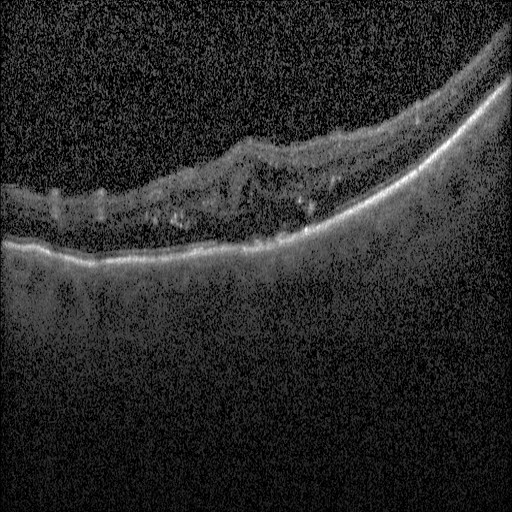 Impression: diabetic macular edema (DME).